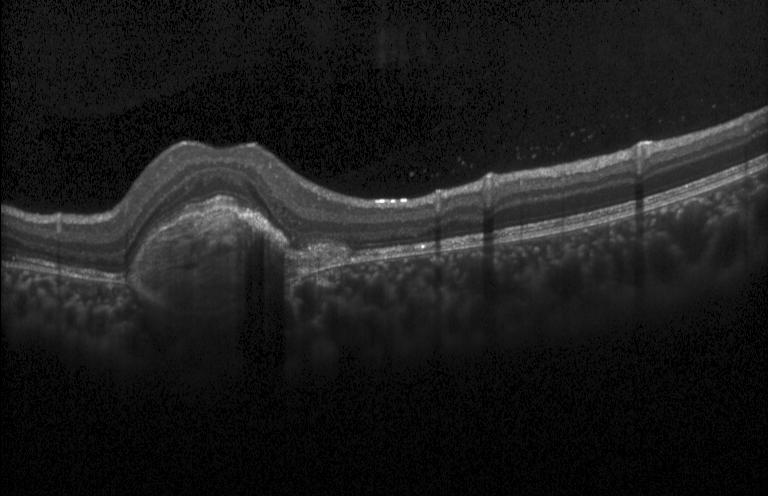

Acquired on a Heidelberg Spectralis. Spectral-domain OCT. OCT B-scan. Through the macula.
Diagnosis: a choroidal neovascular membrane.